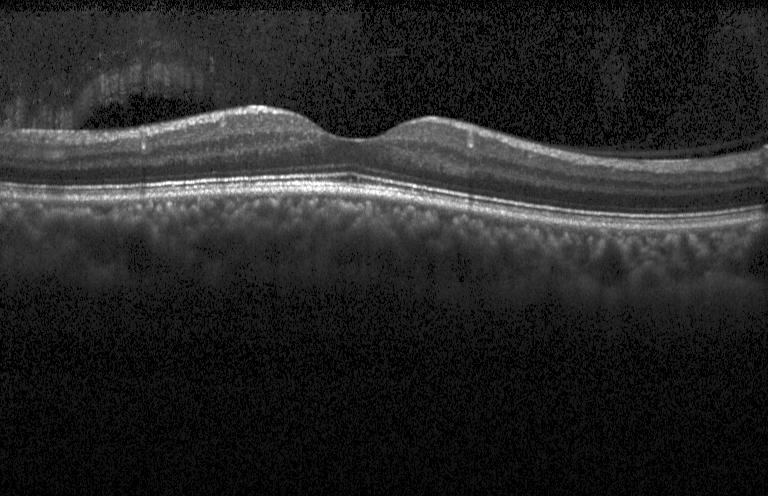

Fovea-centered; OCT B-scan. Finding: no choroidal neovascularization, no diabetic macular edema, and no drusen.